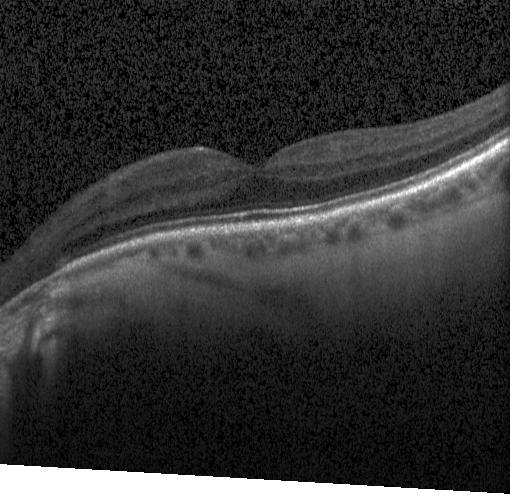 Through the macula · retinal OCT cross-section · acquired on a Heidelberg Spectralis · spectral-domain OCT.
The scan shows no CNV, no DME, and no drusen.